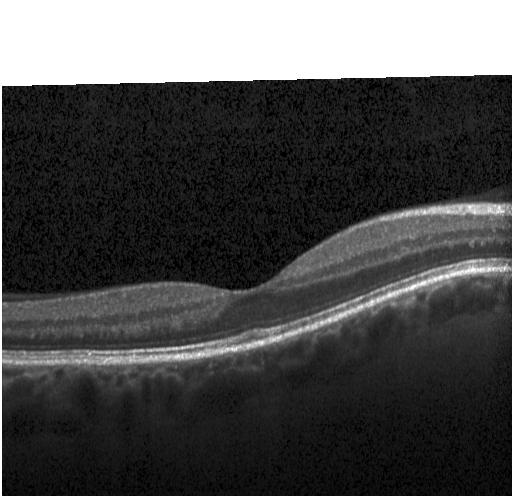 Optical coherence tomography scan. Dx: no evidence of choroidal neovascularization, diabetic macular edema, or drusen.